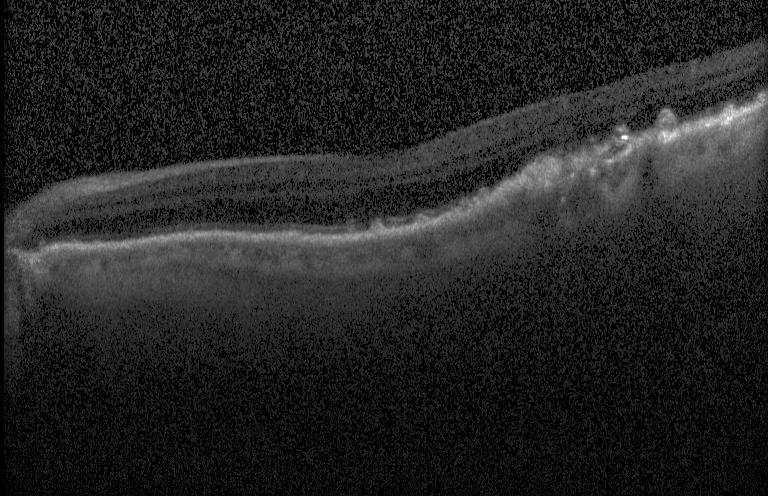

Optical coherence tomography scan, acquired on a Heidelberg Spectralis, spectral-domain OCT, through the macula
Diagnosis: choroidal neovascularization.